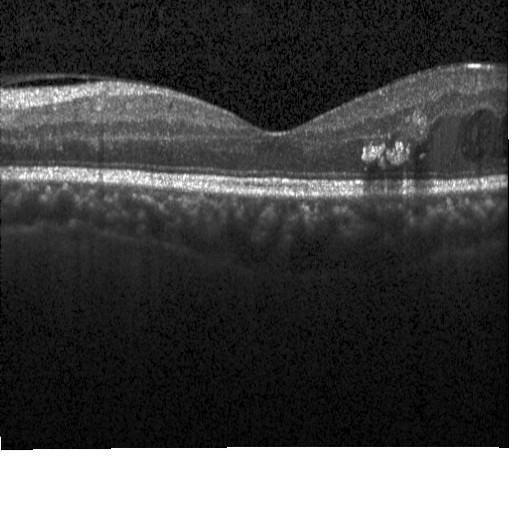 SD-OCT. Heidelberg Spectralis. Retinal OCT cross-section. Fovea-centered.
This B-scan demonstrates diabetic macular edema.